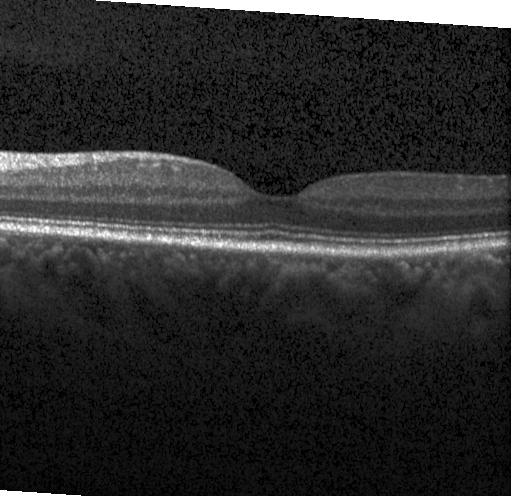 SD-OCT, instrument: Heidelberg Spectralis, retinal OCT cross-section.
The scan shows neither choroidal neovascularization, diabetic macular edema, nor drusen.